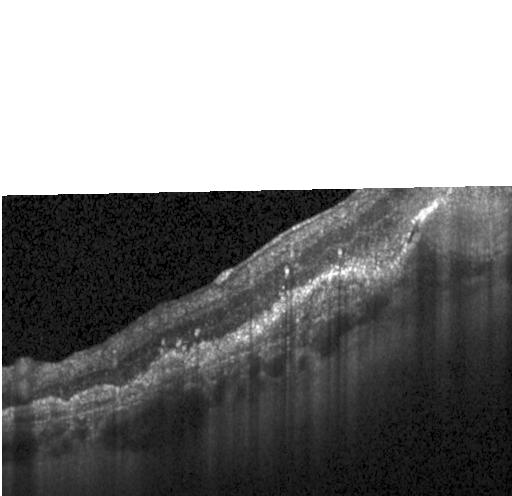

SD-OCT; retinal OCT cross-section; Heidelberg Spectralis OCT system
Assessment: choroidal neovascularization.